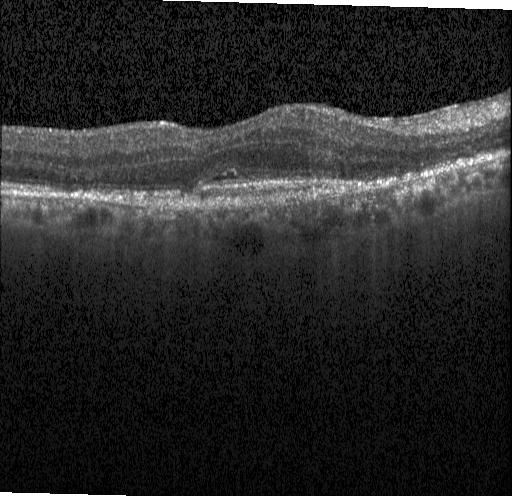
Optical coherence tomography scan; macular scan.
The scan shows choroidal neovascularization (CNV).